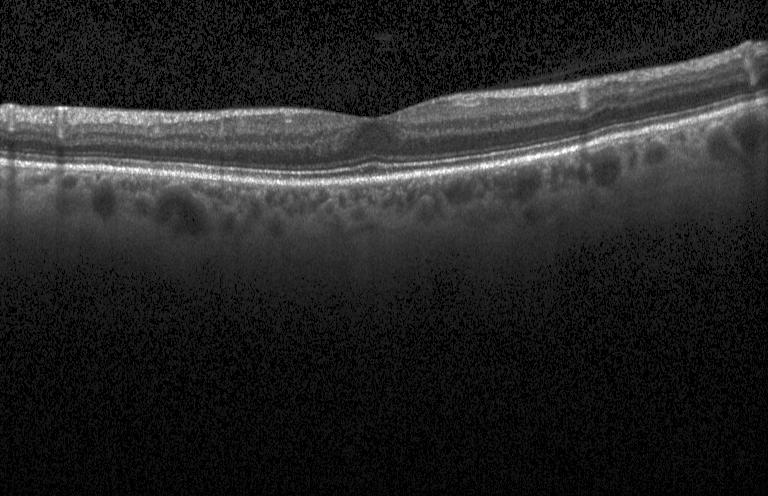
Instrument: Heidelberg Spectralis · retinal OCT B-scan.
Finding: no choroidal neovascularization, no diabetic macular edema, and no drusen.